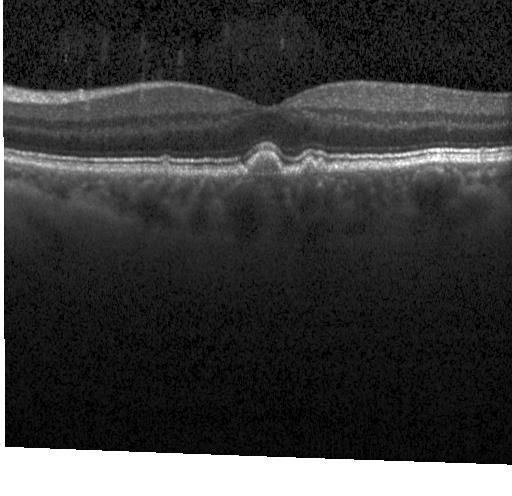

SD-OCT · optical coherence tomography B-scan · fovea-centered · instrument: Heidelberg Spectralis — This B-scan demonstrates sub-RPE drusenoid deposits.